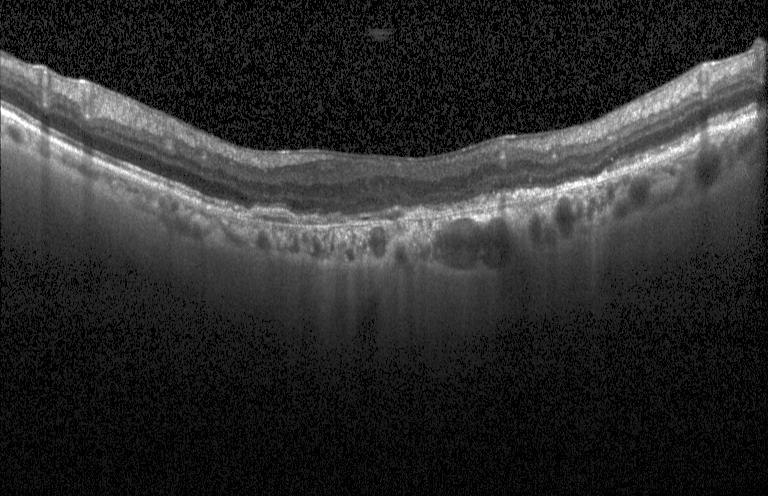

Optical coherence tomography B-scan, instrument: Heidelberg Spectralis, spectral-domain OCT, through the macula.
This B-scan demonstrates CNV.